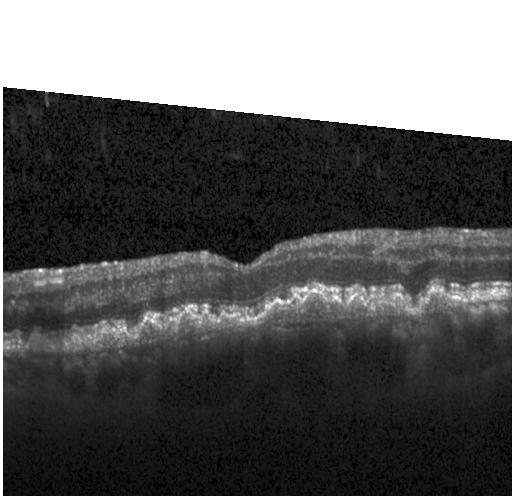
Retinal OCT cross-section showing a choroidal neovascular membrane.